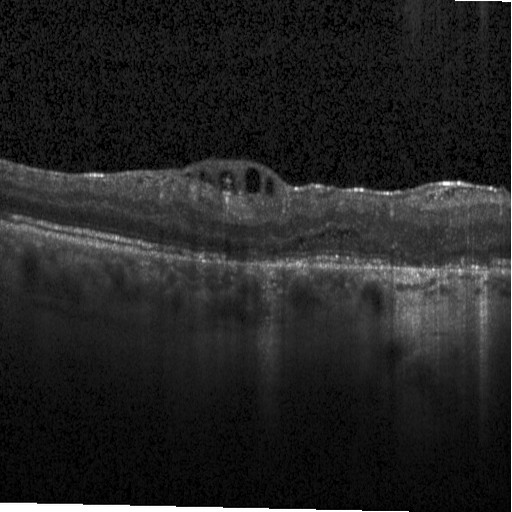 OCT line scan, acquired on a Heidelberg Spectralis
Finding: diabetic macular edema.